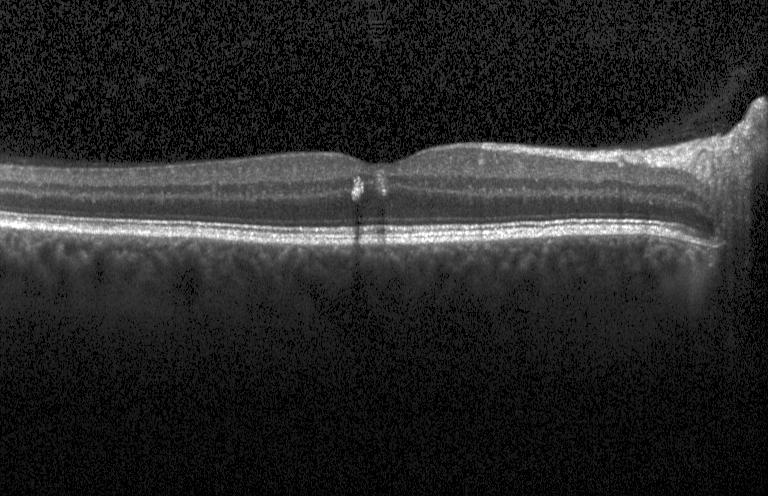 Optical coherence tomography B-scan
Diagnosis: no choroidal neovascularization, diabetic macular edema, or drusen.